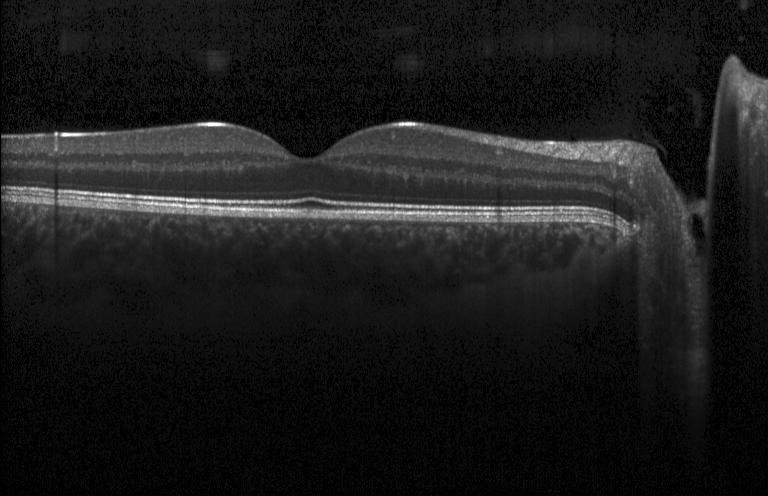
Heidelberg Spectralis; optical coherence tomography scan; spectral-domain optical coherence tomography — Diagnosis: no choroidal neovascularization, no diabetic macular edema, and no drusen.